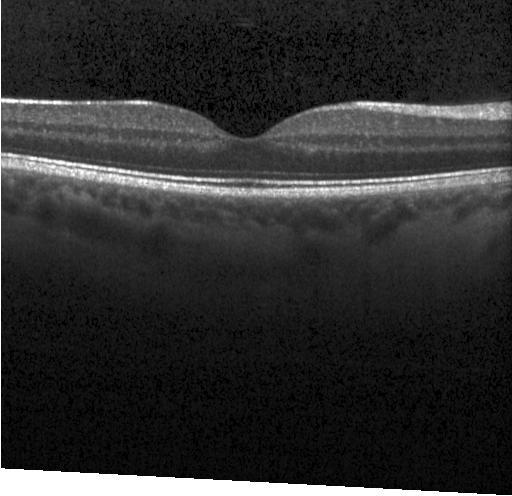 Macular scan · retinal OCT cross-section — Macular OCT: neither CNV, DME, nor drusen.